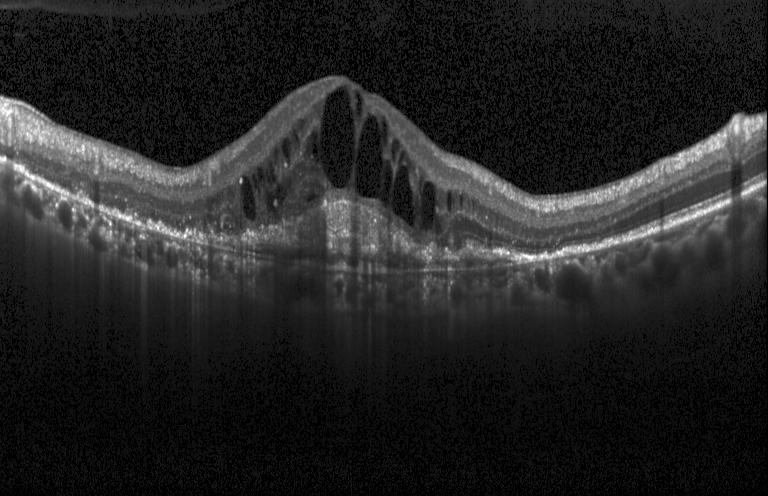 Diagnosis: CNV.